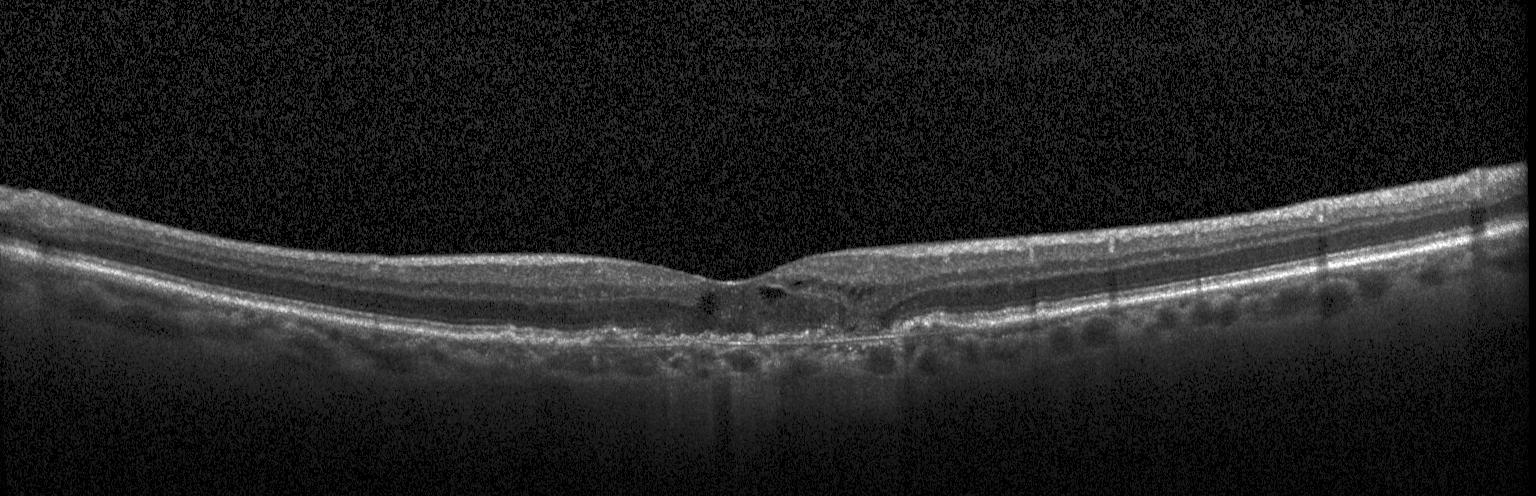

Retinal OCT cross-section showing choroidal neovascularization (CNV).